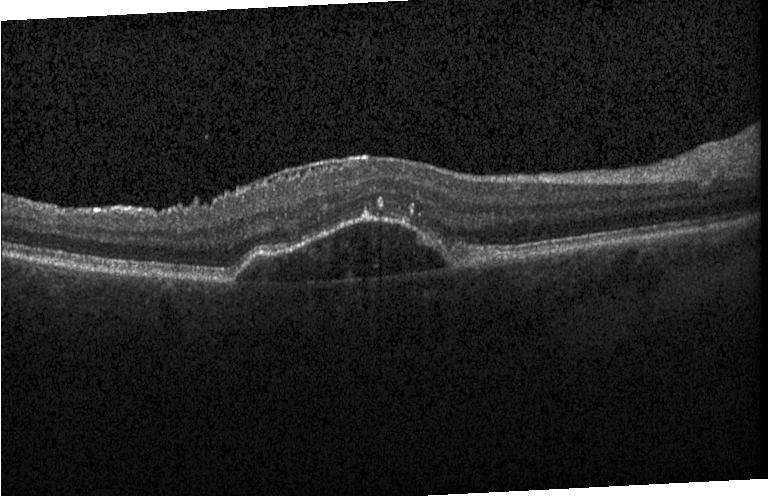

OCT line scan
Impression: choroidal neovascularization (CNV).